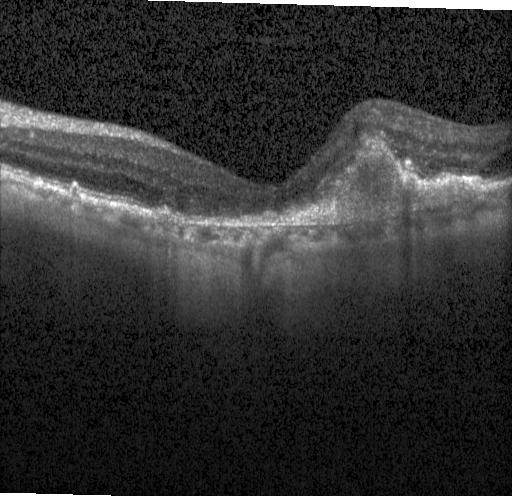

Retinal OCT cross-section. Spectral-domain OCT. Fovea-centered. Acquired on a Heidelberg Spectralis — The scan shows a choroidal neovascular membrane.